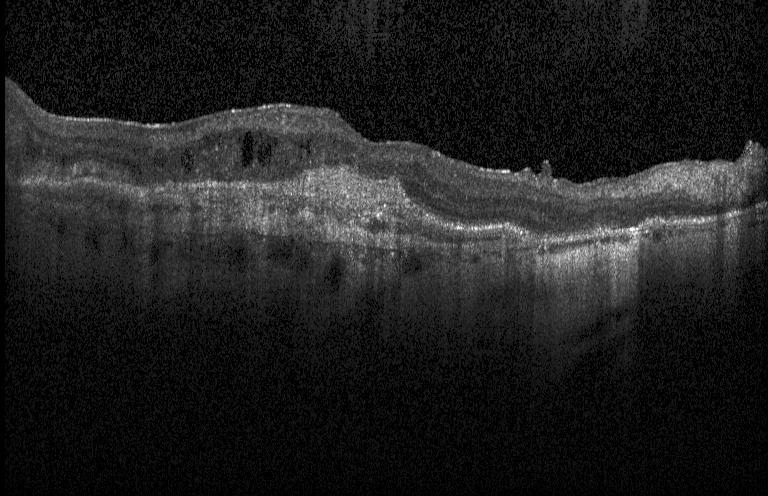
Retinal OCT cross-section — Finding: a choroidal neovascular membrane.